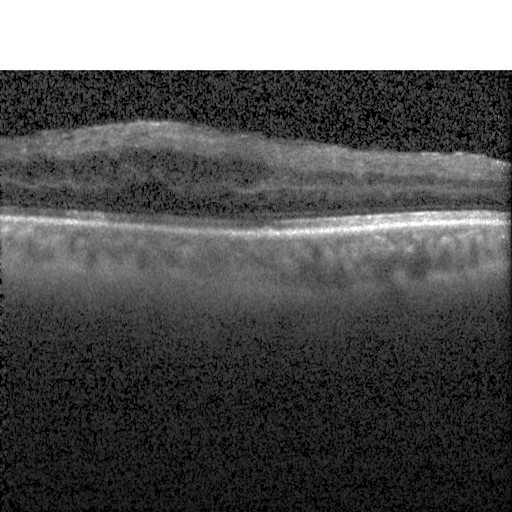 Retinal OCT cross-section showing DME.